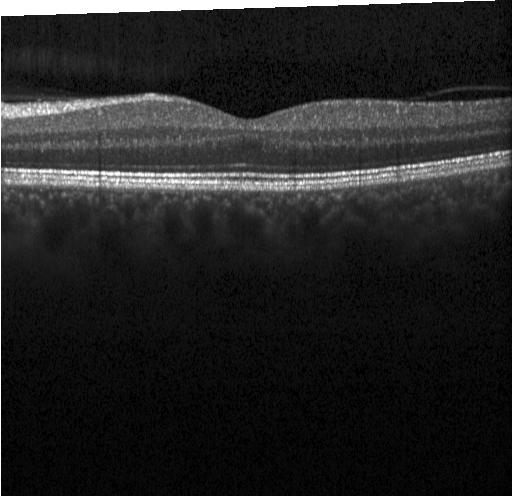 Fovea-centered, optical coherence tomography scan, spectral-domain optical coherence tomography.
OCT finding: neither CNV, DME, nor drusen.